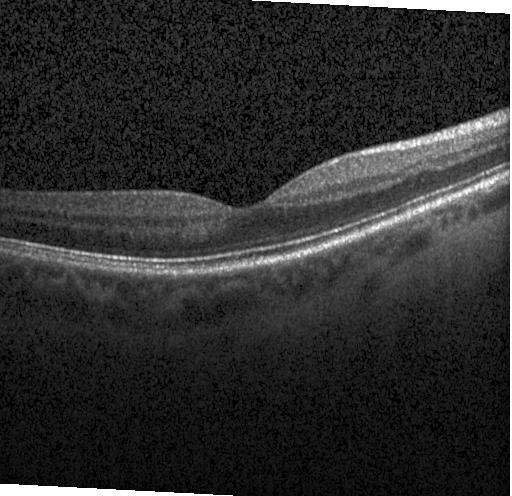

This B-scan demonstrates no choroidal neovascularization, no diabetic macular edema, and no drusen.